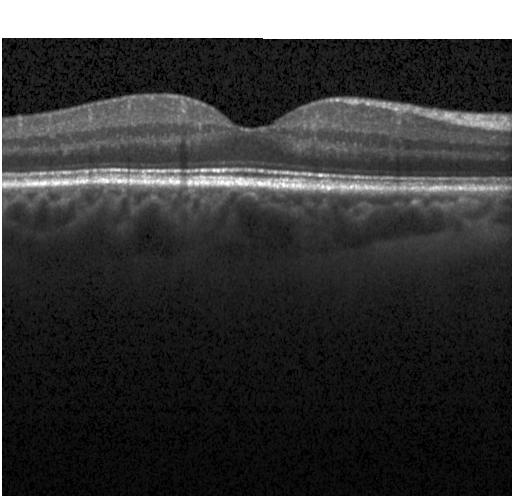

OCT B-scan. Finding: no choroidal neovascularization, no diabetic macular edema, and no drusen.